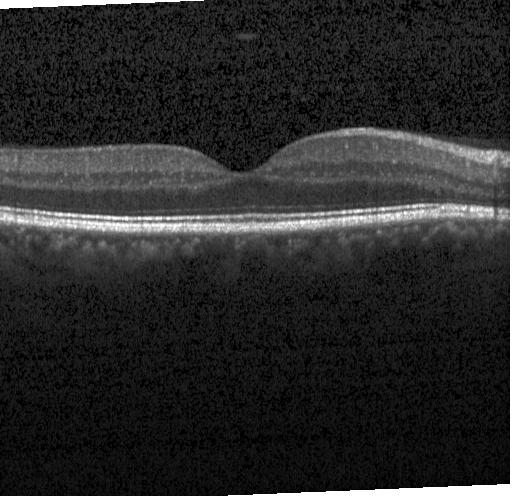 Assessment: no CNV, no DME, and no drusen.